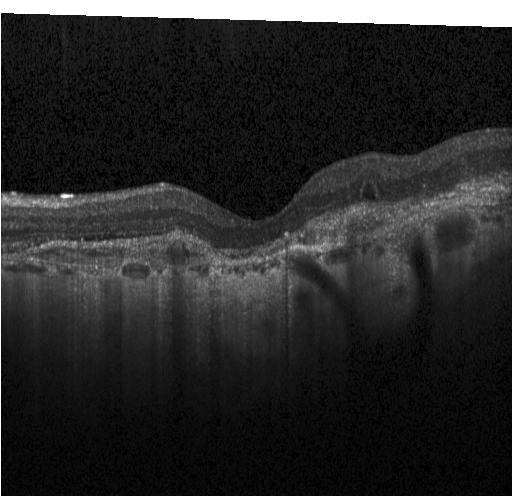
Retinal OCT cross-section, Heidelberg Spectralis, macular scan. Dx: a choroidal neovascular membrane.